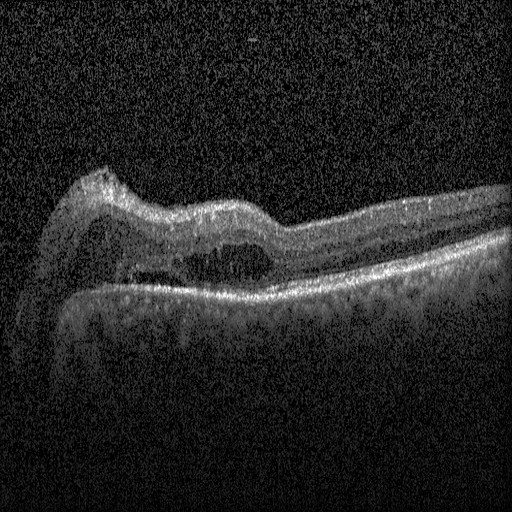

Impression: diabetic macular edema.